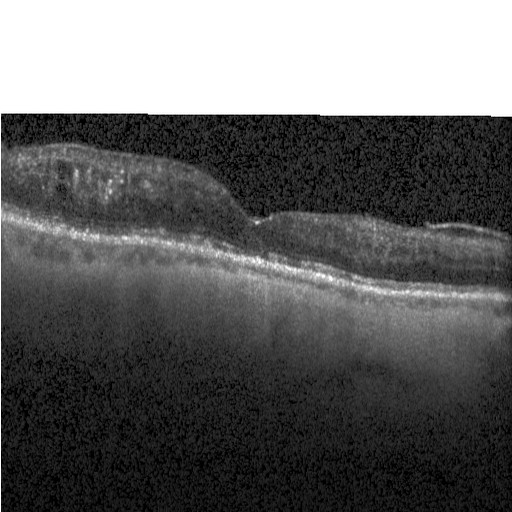
DME.